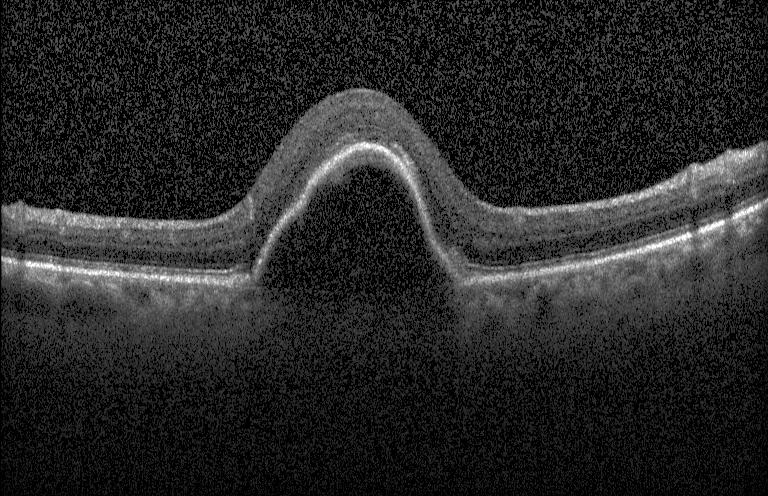
Macular scan; acquired on a Heidelberg Spectralis; OCT B-scan; SD-OCT — Impression: CNV.